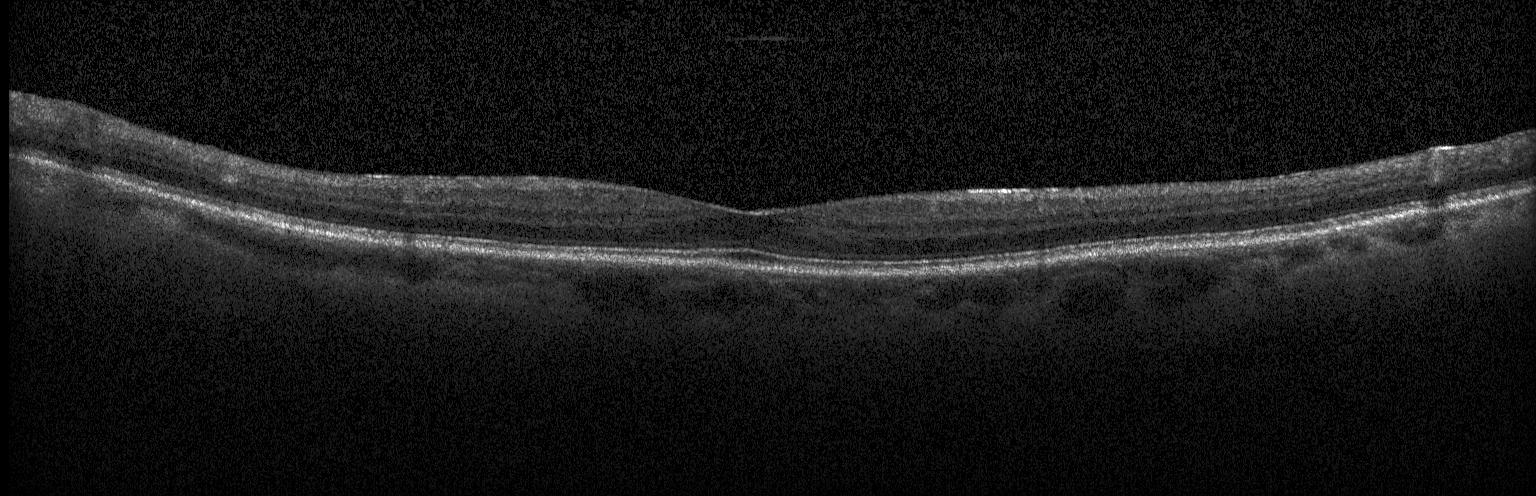 Heidelberg Spectralis, SD-OCT, OCT line scan — Impression: neither CNV, DME, nor drusen.